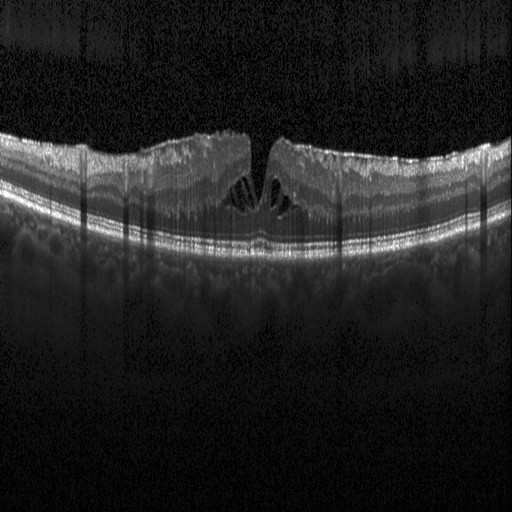 Optical coherence tomography scan. Heidelberg Spectralis OCT system. SD-OCT. Through the macula
Impression: diabetic macular edema (DME).